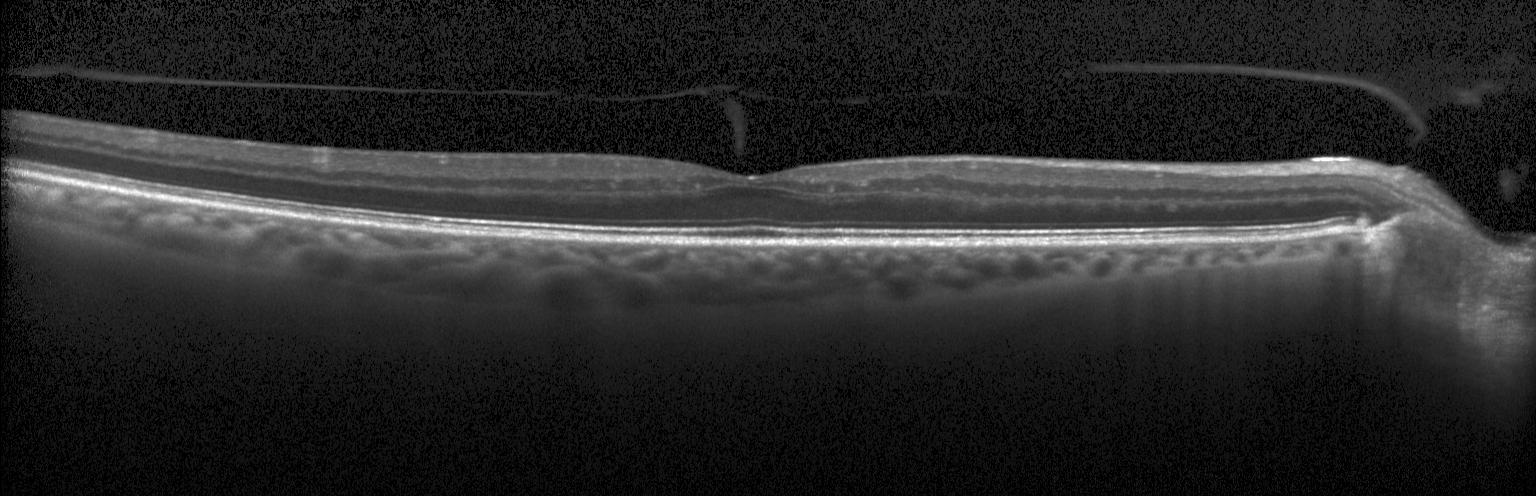

Optical coherence tomography scan; horizontal scan through the fovea
Impression: no choroidal neovascularization, no diabetic macular edema, and no drusen.